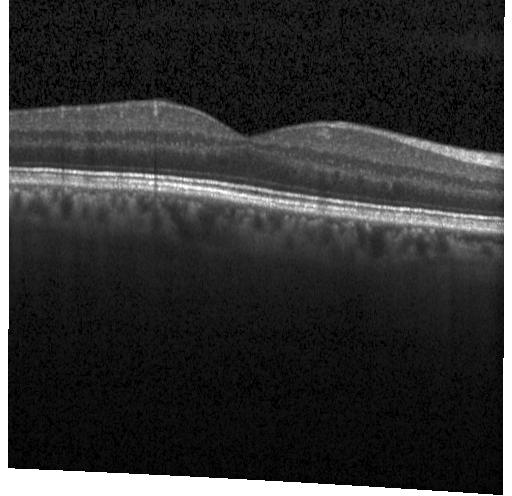

Assessment: no CNV, no DME, and no drusen.